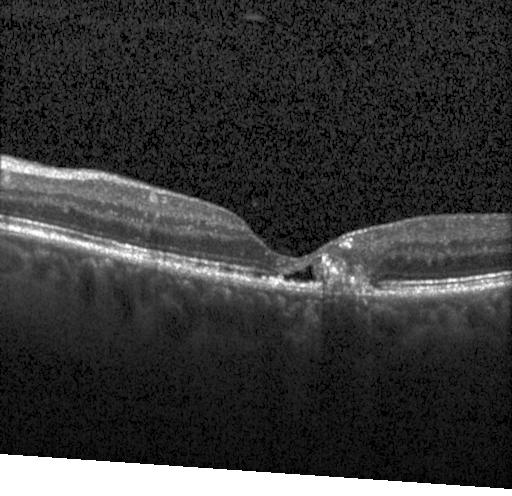
OCT B-scan.
Dx: choroidal neovascularization.